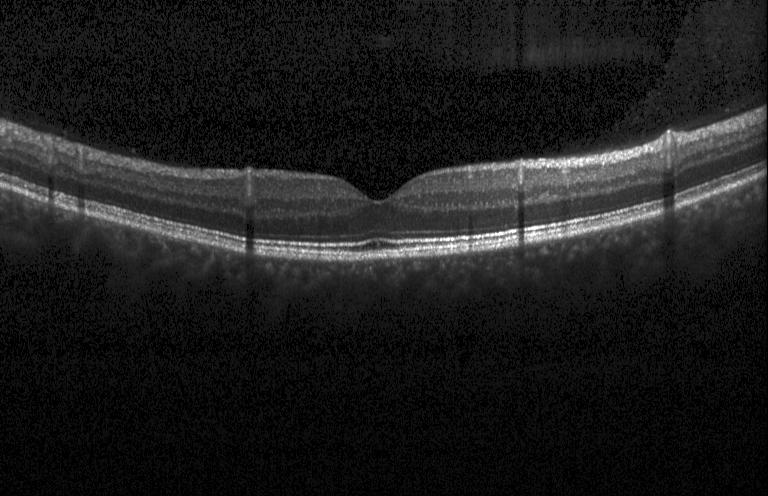 Macular OCT demonstrating no CNV, no DME, and no drusen.